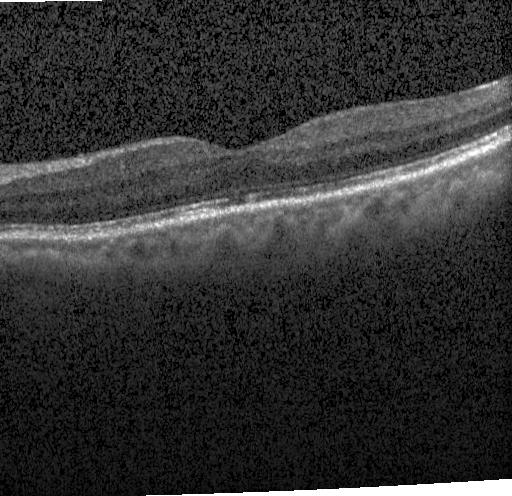 Diagnosis: no choroidal neovascularization, no diabetic macular edema, and no drusen.